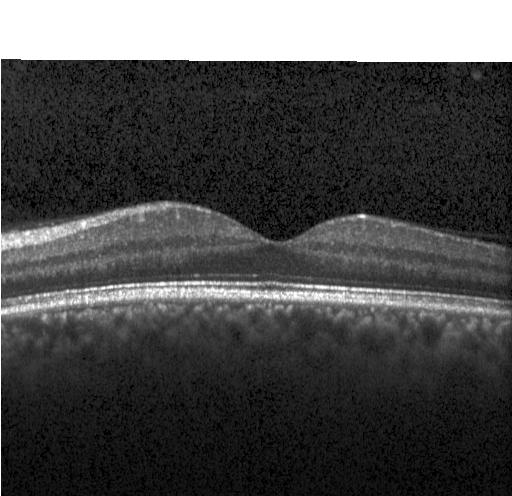

Impression: no choroidal neovascularization, no diabetic macular edema, and no drusen.